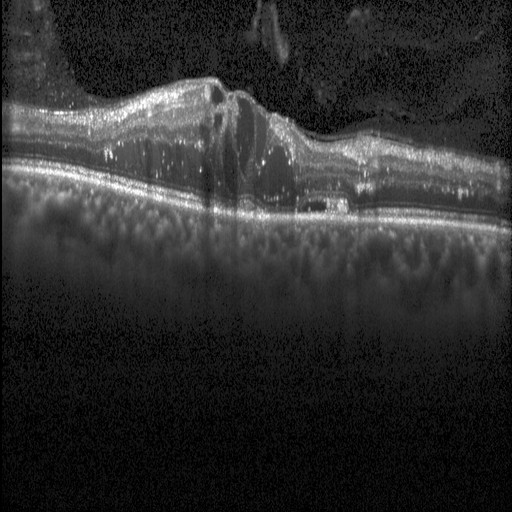
Retinal OCT cross-section.
Finding: diabetic macular edema.